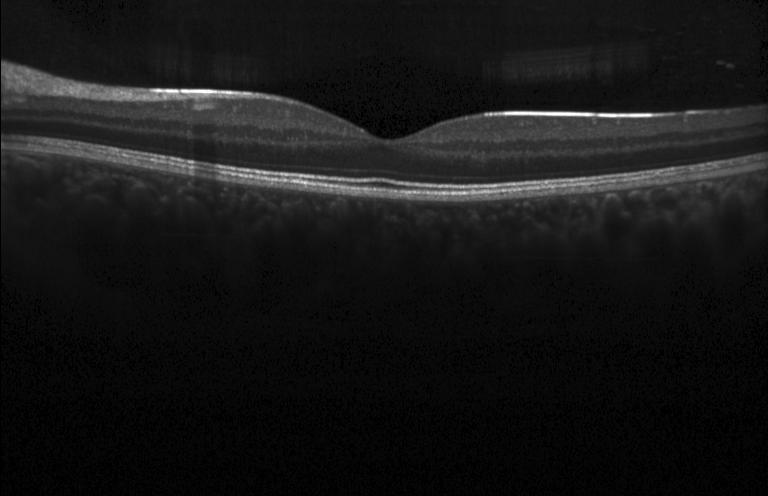
Spectral-domain OCT B-scan: no evidence of choroidal neovascularization, diabetic macular edema, or drusen.